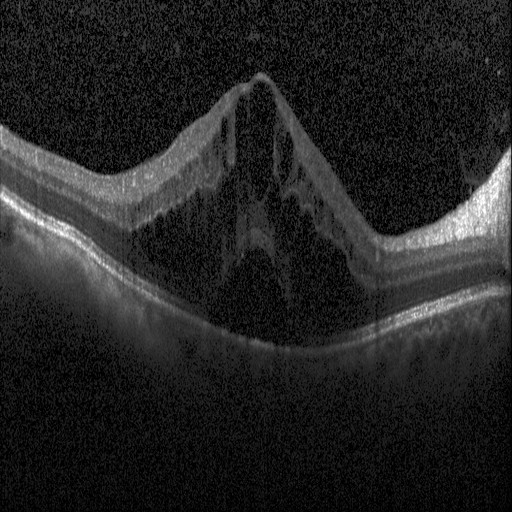

DME.